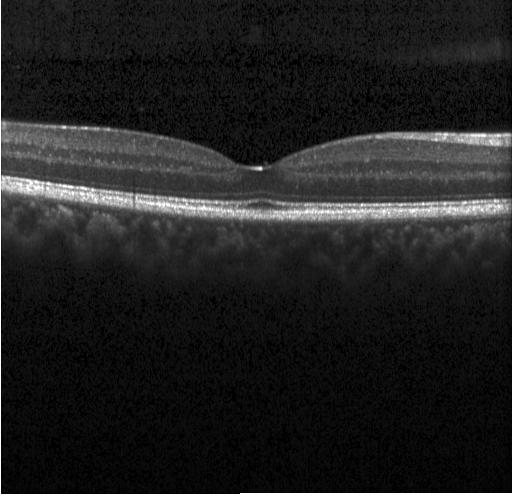

SD-OCT, centered on the fovea, retinal OCT B-scan. The scan shows no CNV, no DME, and no drusen.